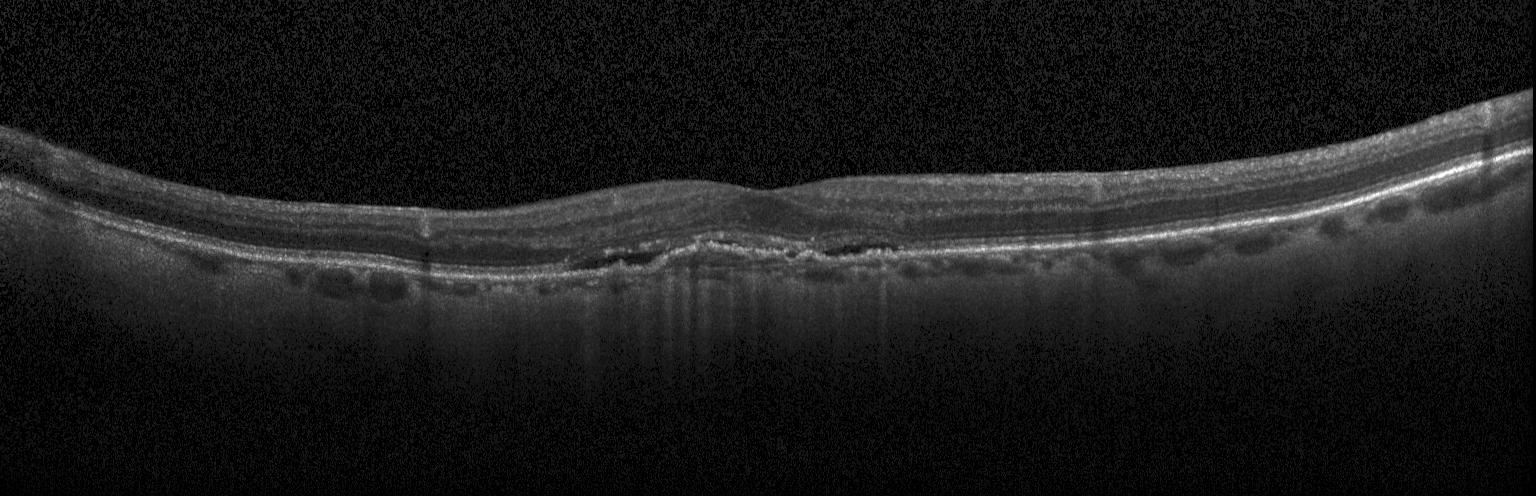
OCT B-scan, Heidelberg Spectralis OCT system.
Finding: choroidal neovascularization.